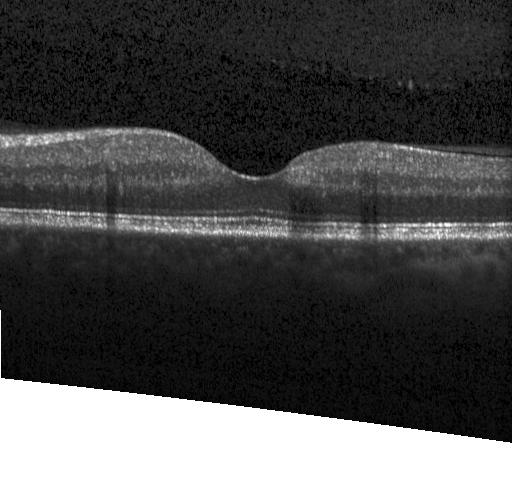

Diagnosis: neither choroidal neovascularization, diabetic macular edema, nor drusen.